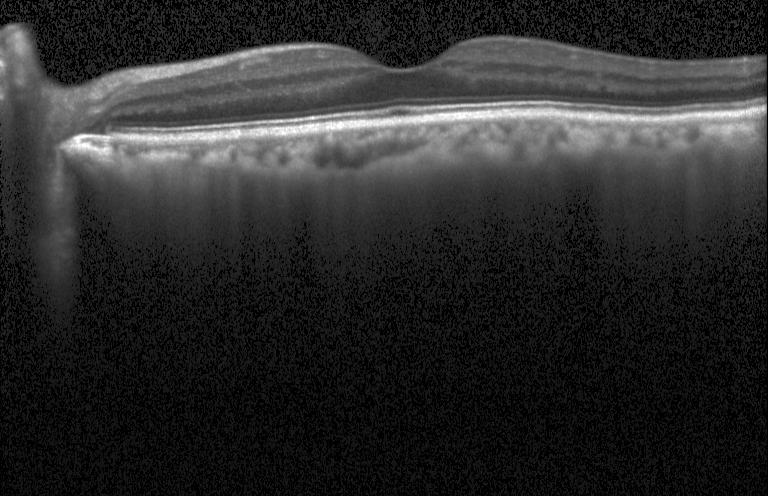
Retinal OCT cross-section showing no evidence of CNV, DME, or drusen.